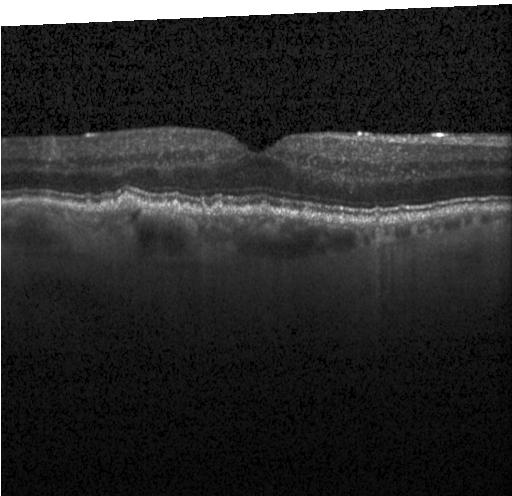
OCT scan showing multiple drusen.